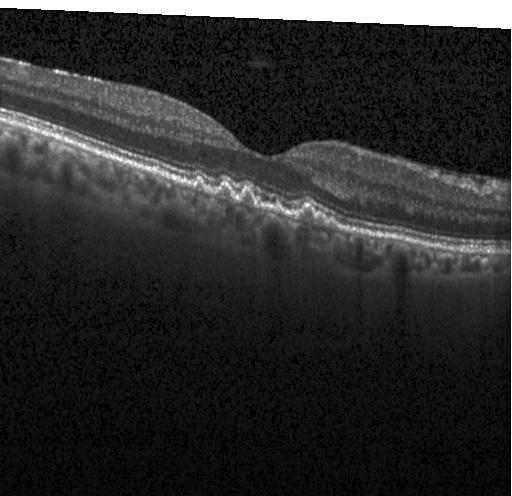

Optical coherence tomography scan. Impression: drusen.